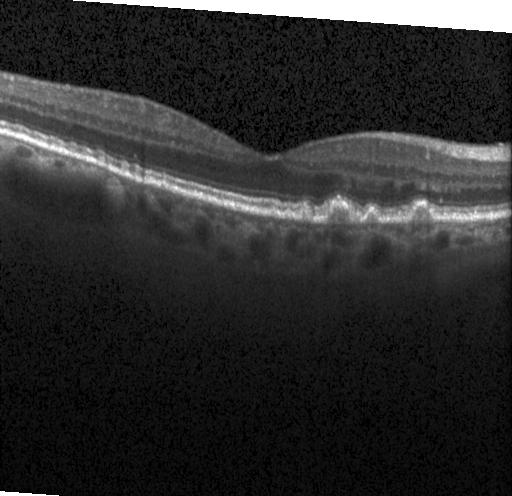 Impression: sub-RPE drusenoid deposits.